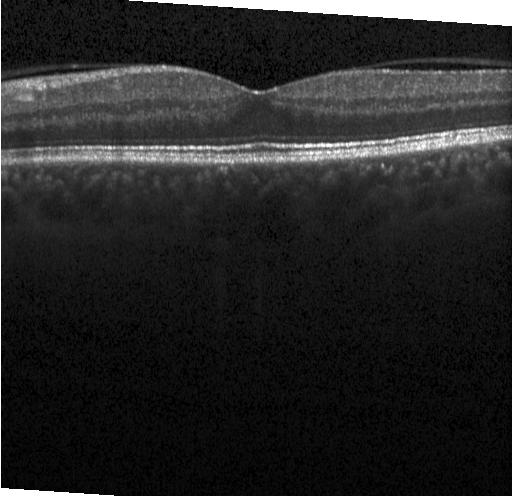
Retinal OCT cross-section, spectral-domain OCT, macular scan. The scan shows neither choroidal neovascularization, diabetic macular edema, nor drusen.